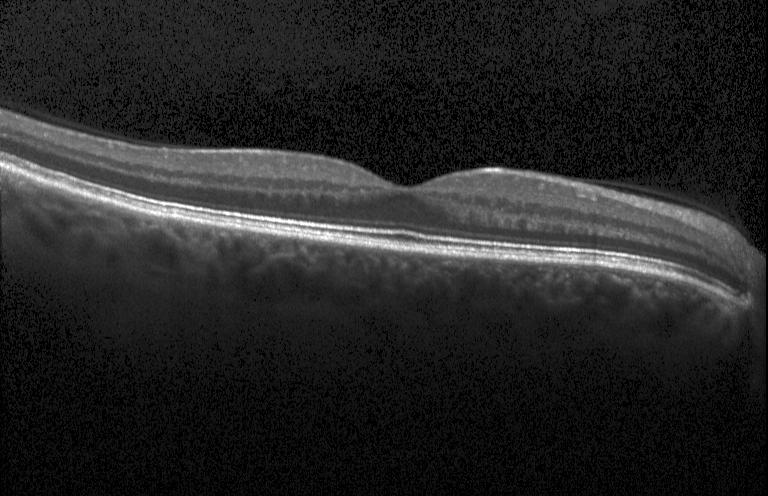
Dx: neither choroidal neovascularization, diabetic macular edema, nor drusen.